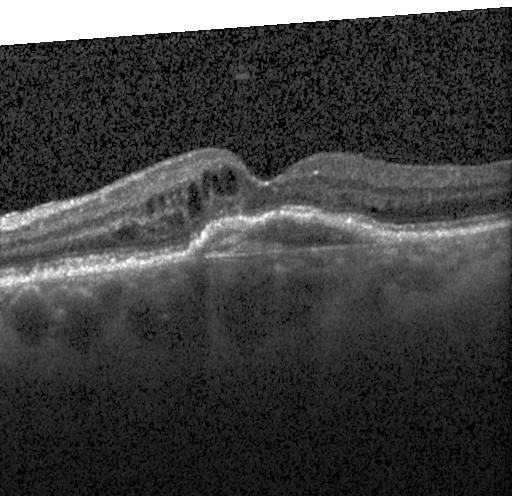 OCT B-scan; Heidelberg Spectralis OCT system.
Assessment: CNV.